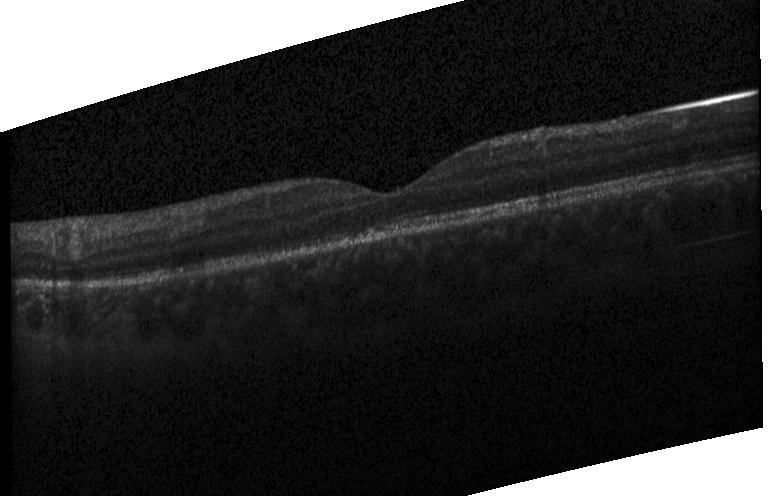
Retinal OCT B-scan, Heidelberg Spectralis OCT system
Neither choroidal neovascularization, diabetic macular edema, nor drusen.